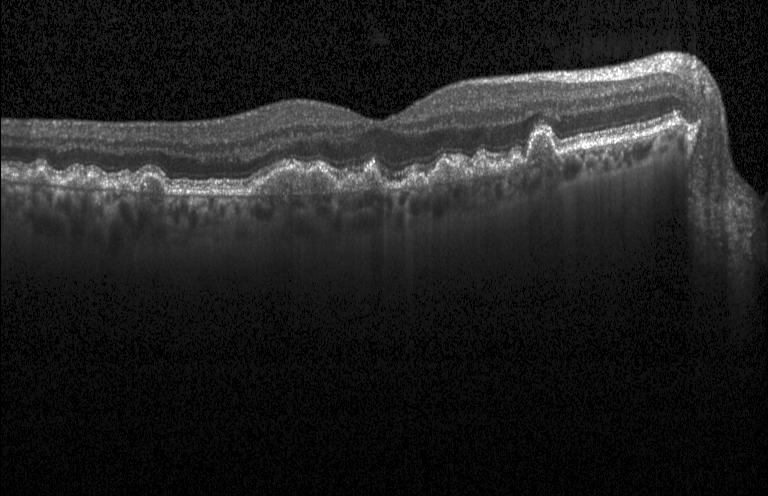

Optical coherence tomography B-scan, spectral-domain optical coherence tomography — Multiple drusen.